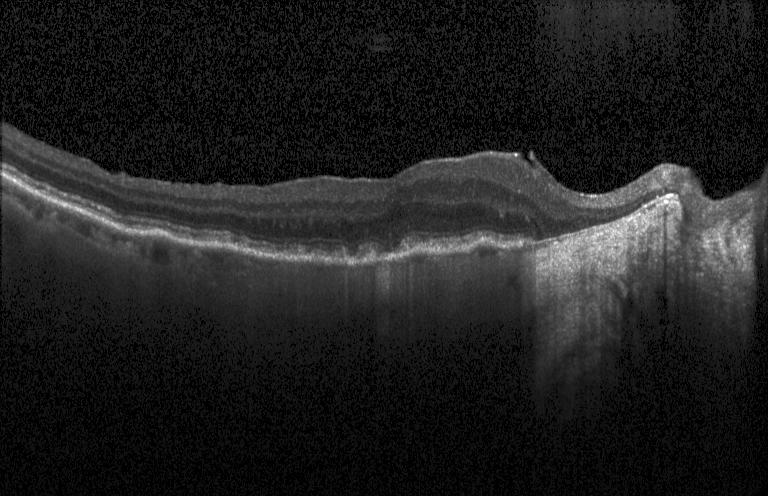
Through the macula. Retinal OCT B-scan — Dx: multiple drusen.